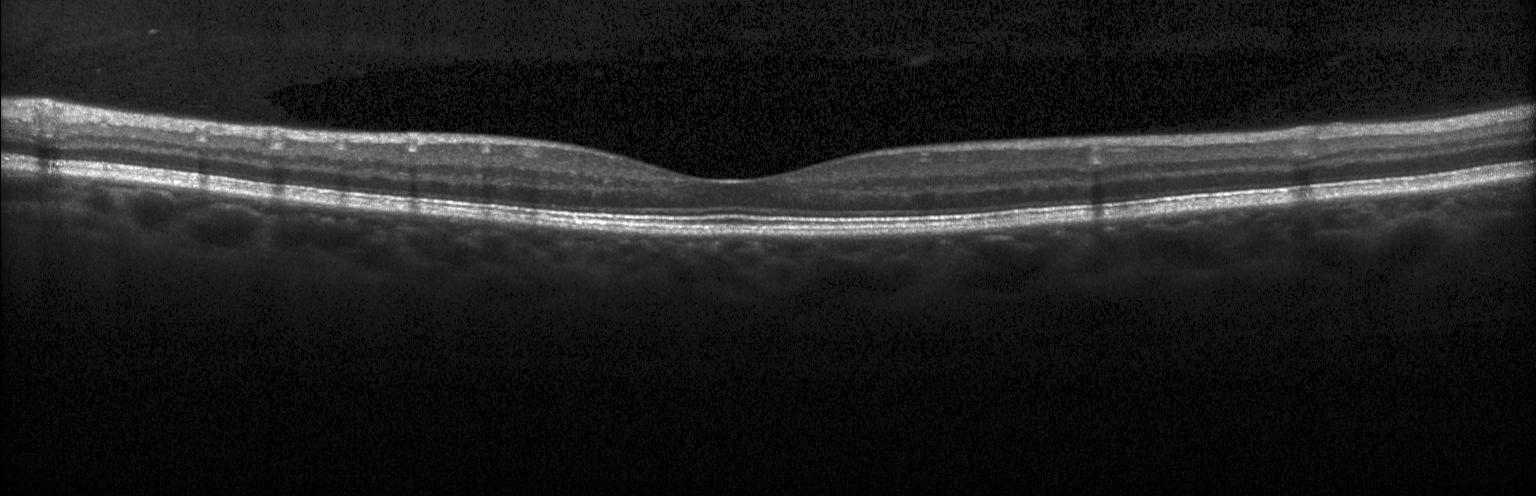 Optical coherence tomography B-scan — Diagnosis: no CNV, no DME, and no drusen.